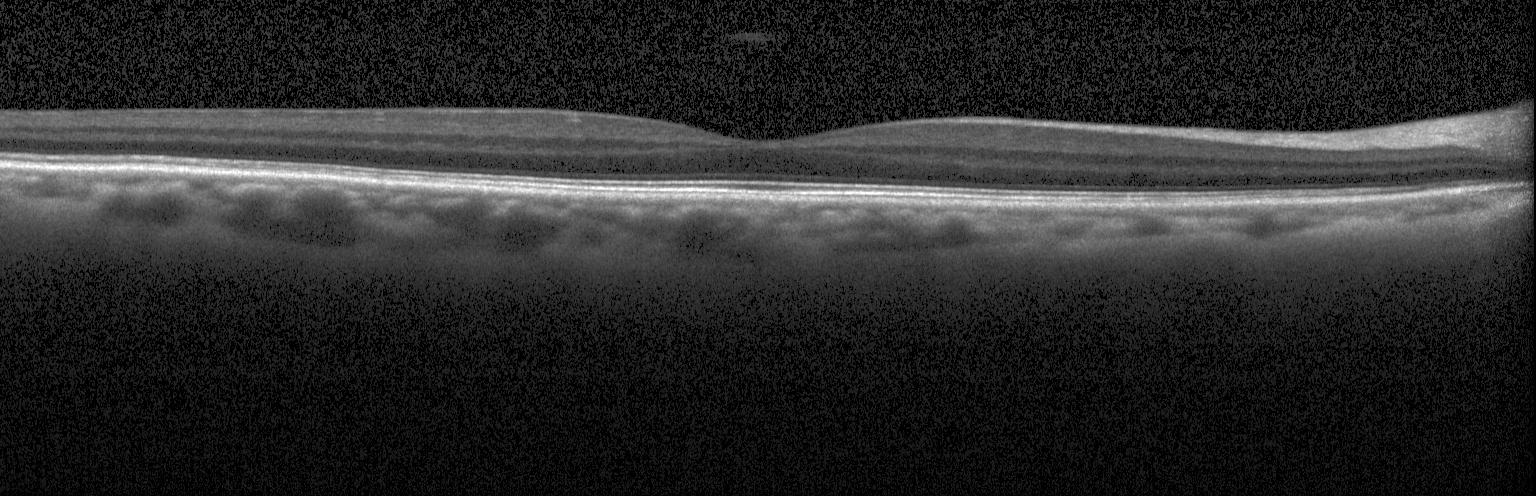
Impression: neither CNV, DME, nor drusen.